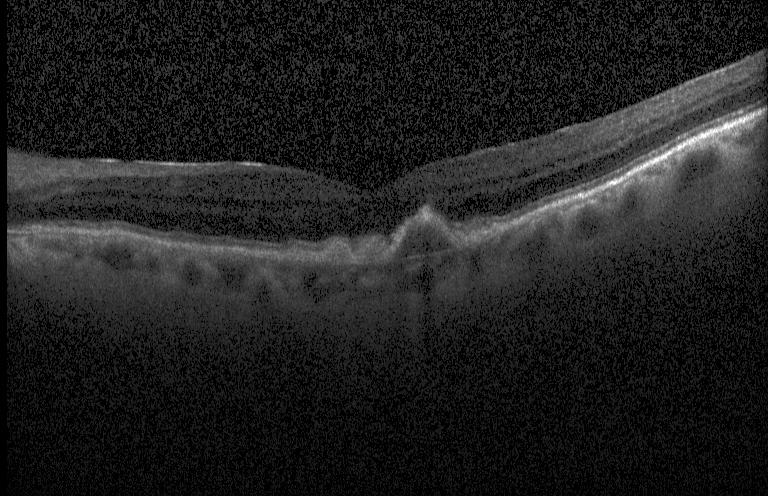 Drusen.